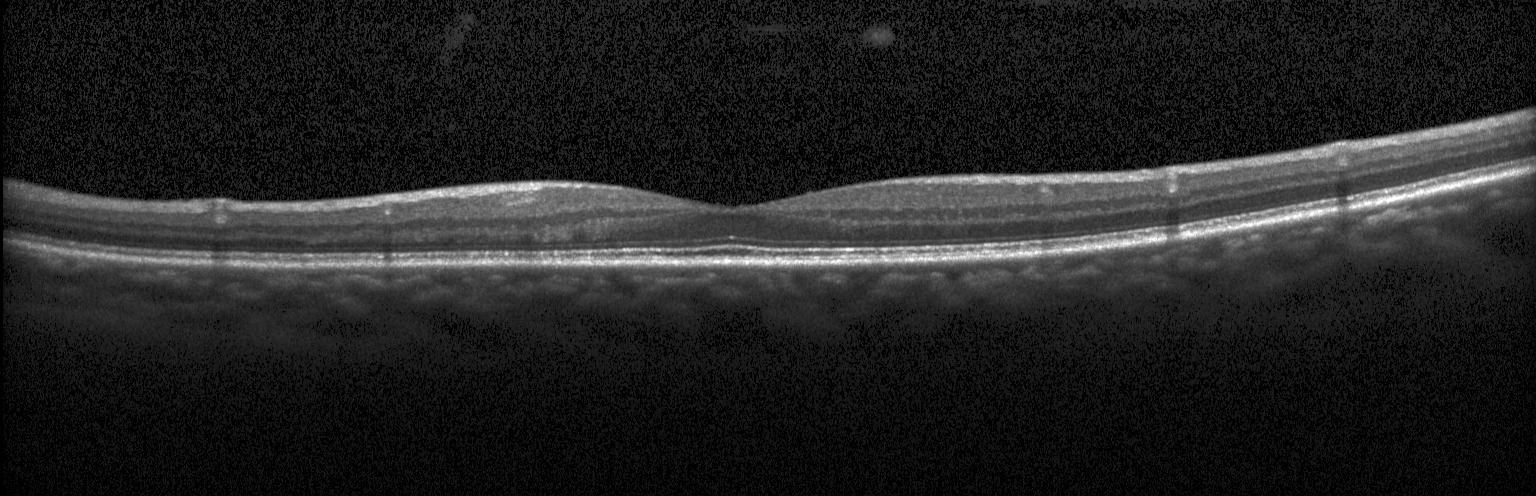

OCT line scan — Finding: no CNV, DME, or drusen.